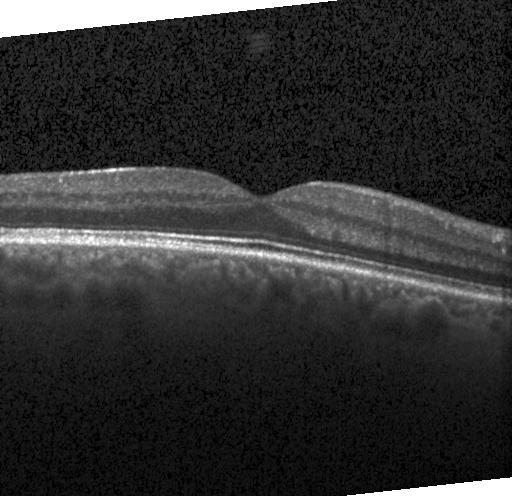

OCT scan showing no choroidal neovascularization, no diabetic macular edema, and no drusen.